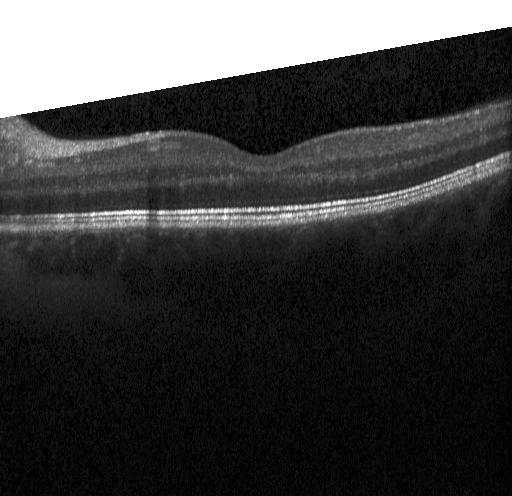

Macular scan; optical coherence tomography scan.
Diagnosis: neither choroidal neovascularization, diabetic macular edema, nor drusen.